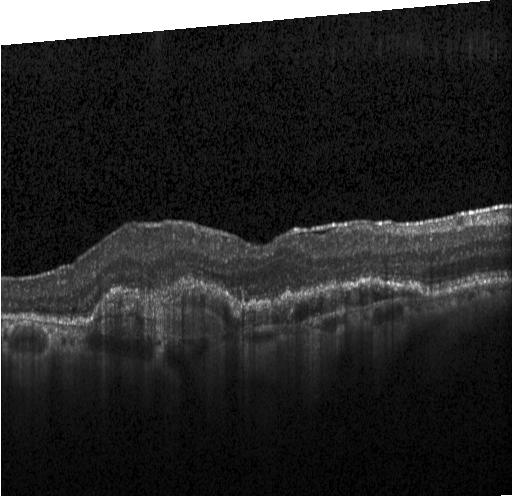

Optical coherence tomography B-scan · fovea-centered — A choroidal neovascular membrane.